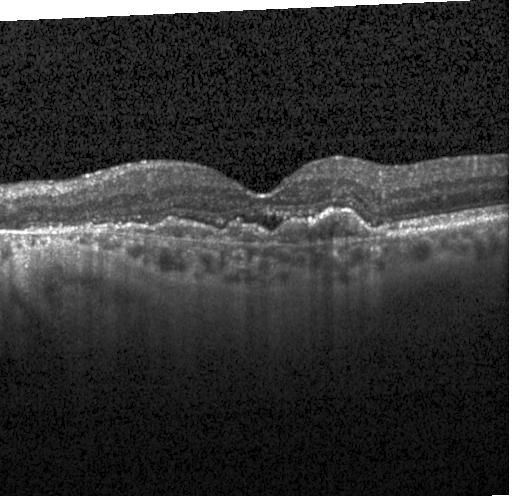 Finding: CNV.